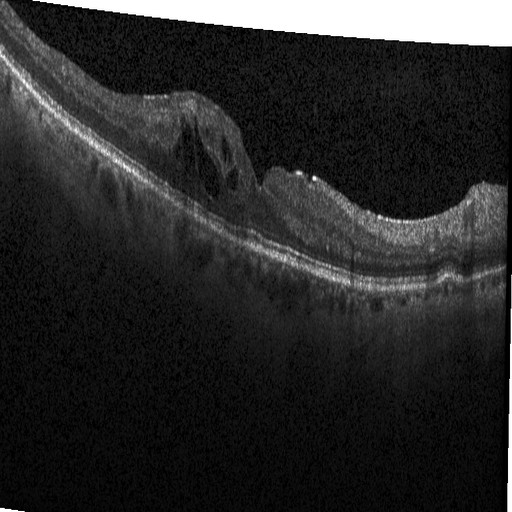

OCT B-scan · Heidelberg Spectralis — Assessment: diabetic macular edema.